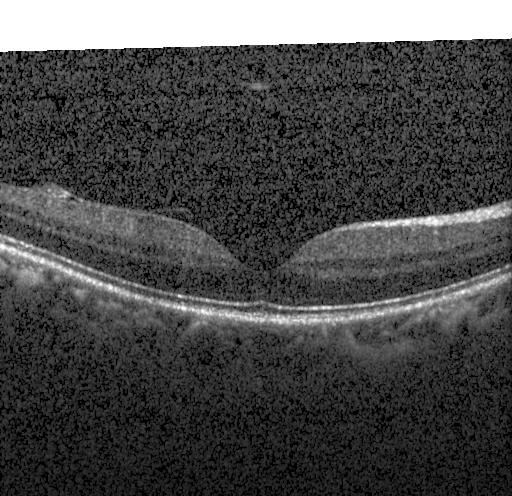 Through the macula. OCT line scan. Heidelberg Spectralis OCT system
Dx: no choroidal neovascularization, diabetic macular edema, or drusen.